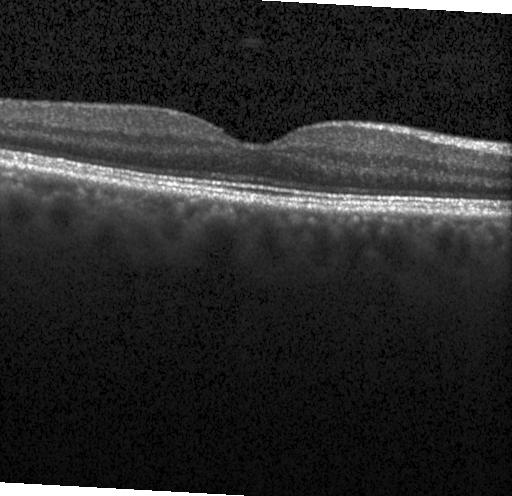 Through the macula · OCT line scan. No CNV, DME, or drusen.